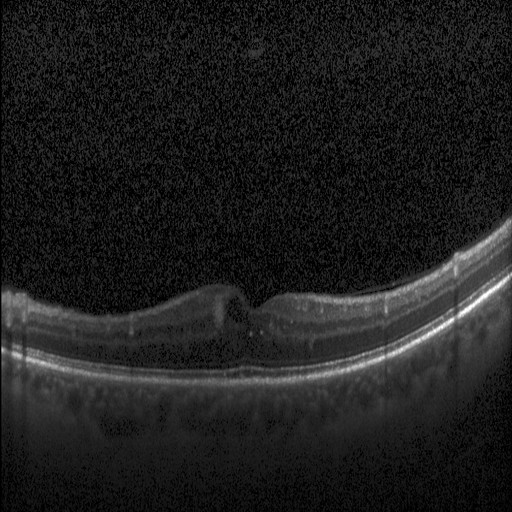

Retinal OCT cross-section.
Impression: DME.